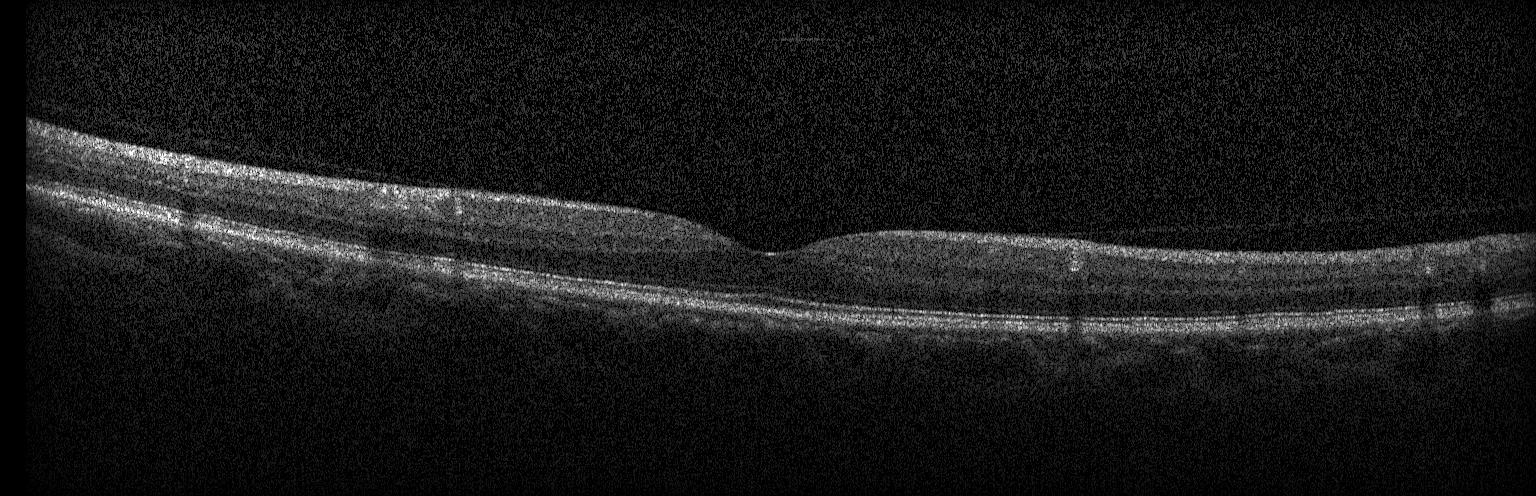

Through the macula; SD-OCT; optical coherence tomography scan. Macular OCT: no choroidal neovascularization, no diabetic macular edema, and no drusen.